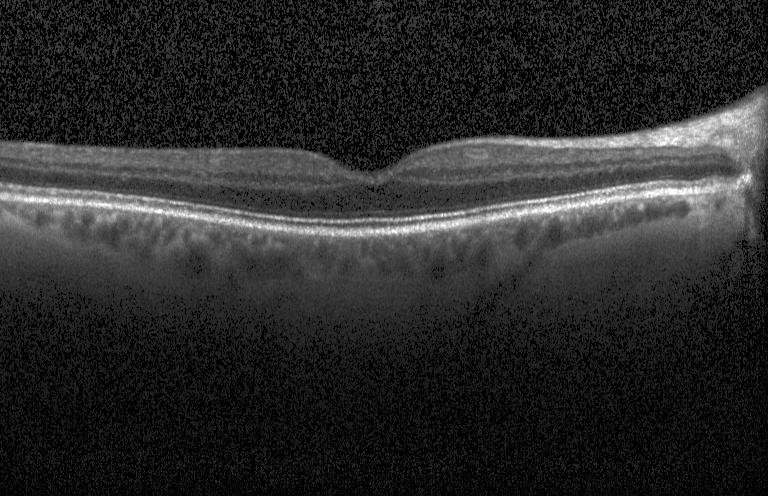

Optical coherence tomography scan · Heidelberg Spectralis · macular scan. The scan shows no evidence of choroidal neovascularization, diabetic macular edema, or drusen.